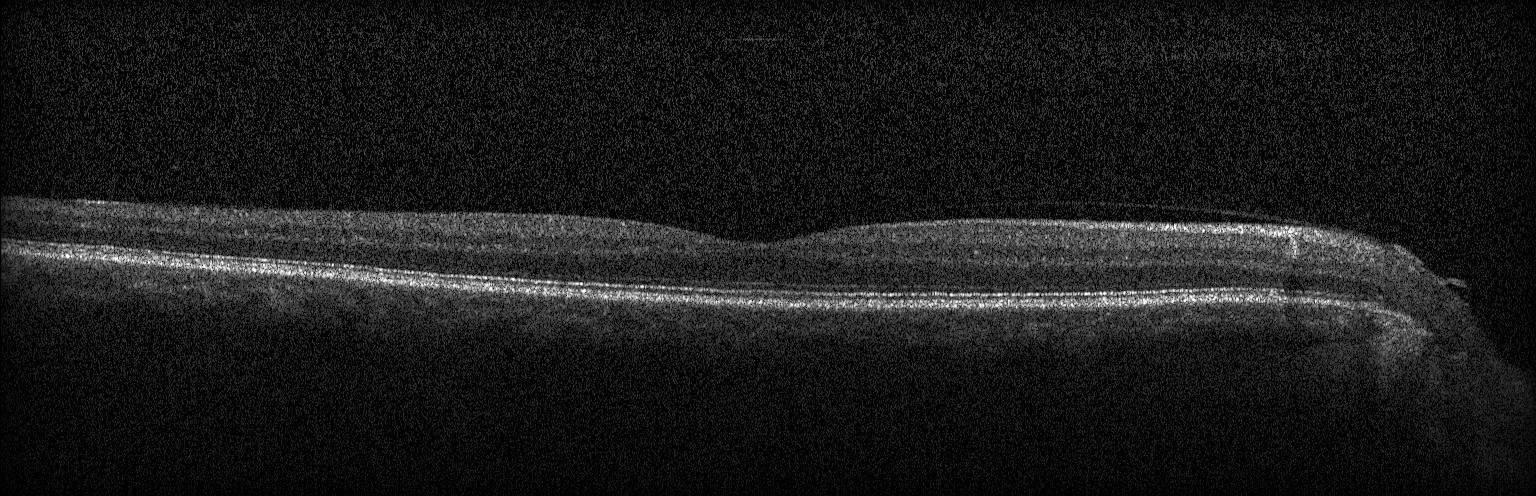
OCT line scan, fovea-centered. This B-scan demonstrates no choroidal neovascularization, diabetic macular edema, or drusen.